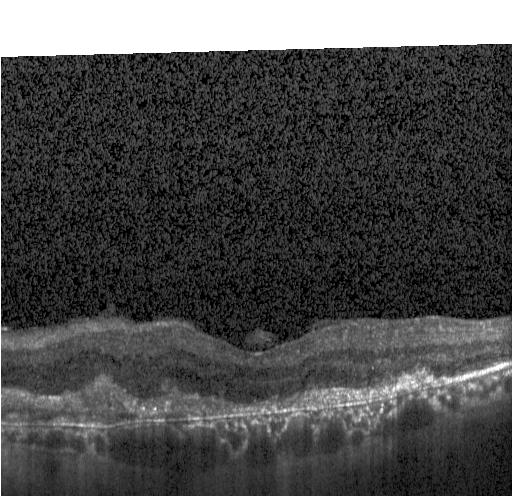
Macular OCT: a choroidal neovascular membrane.